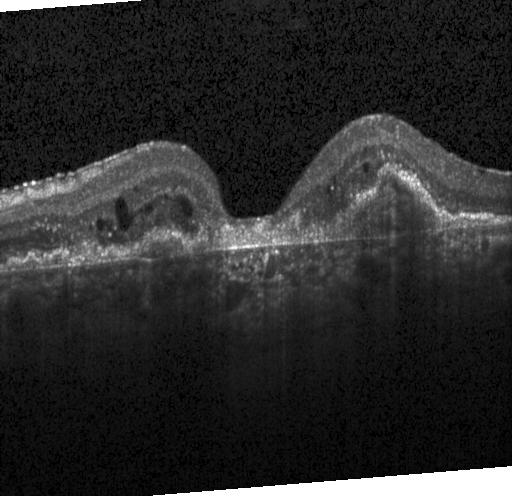
OCT line scan, macular scan.
Assessment: a choroidal neovascular membrane.